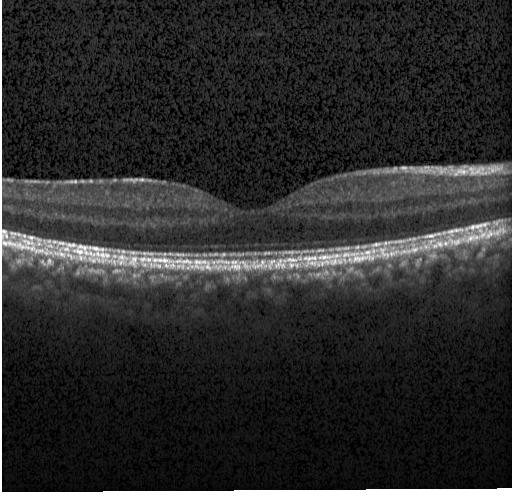
OCT line scan, Heidelberg Spectralis OCT system.
No choroidal neovascularization, diabetic macular edema, or drusen.